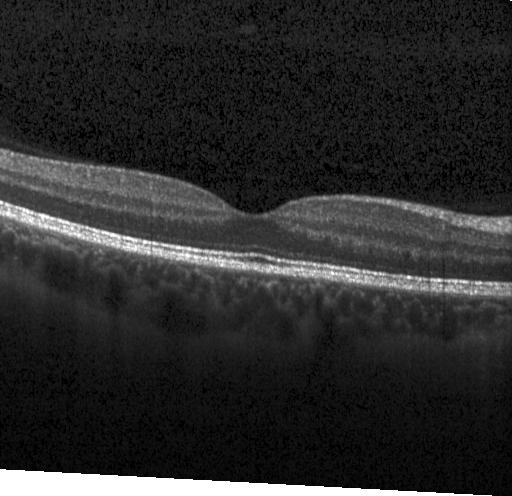
Dx: neither CNV, DME, nor drusen.